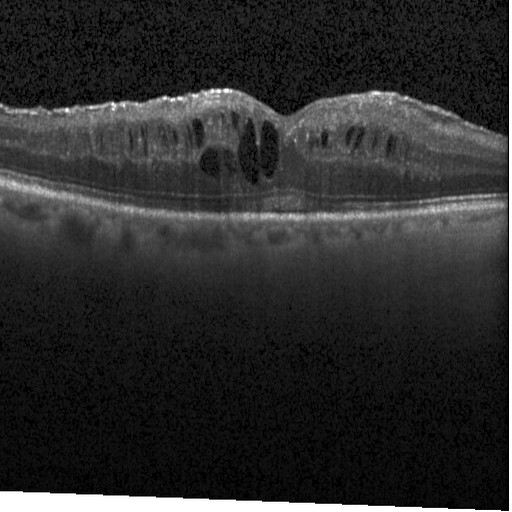
Retinal OCT B-scan · instrument: Heidelberg Spectralis · fovea-centered — Impression: diabetic macular edema (DME).